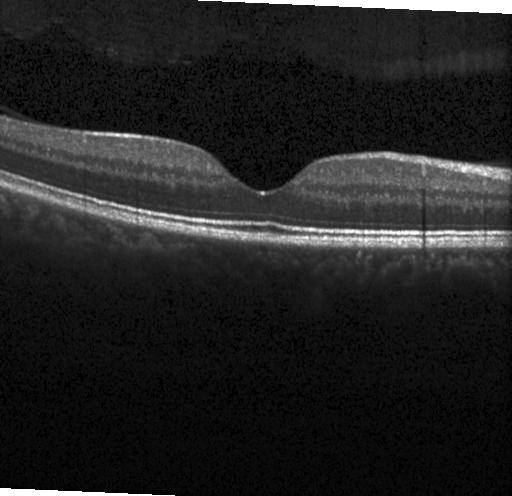
Optical coherence tomography scan. Impression: neither choroidal neovascularization, diabetic macular edema, nor drusen.